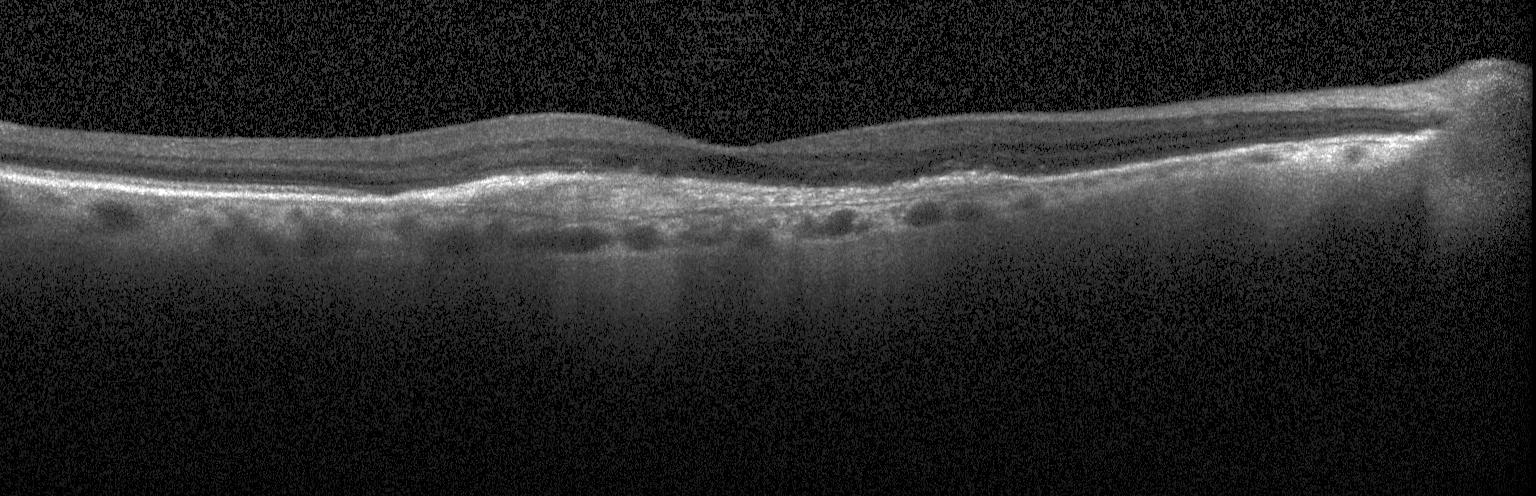 Spectral-domain OCT, Heidelberg Spectralis OCT system, through the macula, optical coherence tomography B-scan.
Diagnosis: choroidal neovascularization.